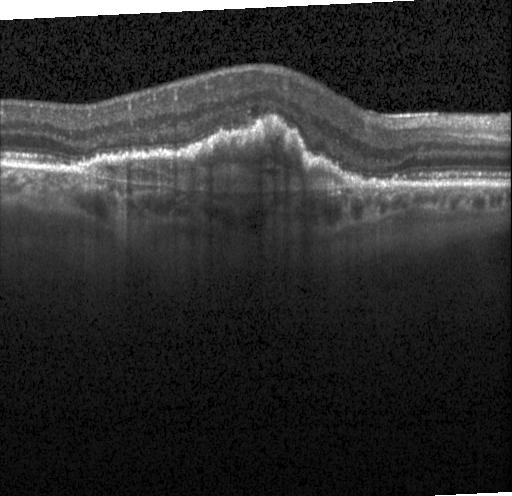 Retinal OCT cross-section — Finding: a choroidal neovascular membrane.